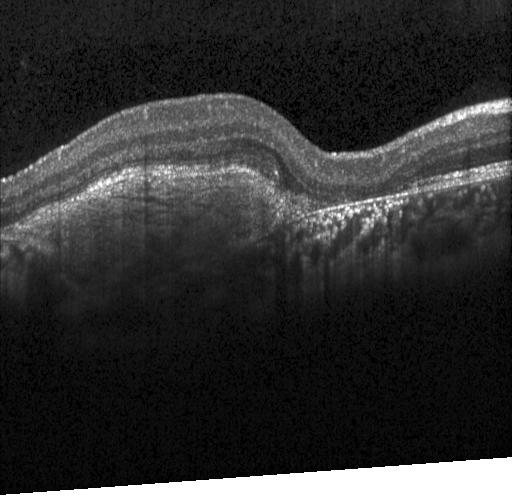
Optical coherence tomography B-scan.
Impression: choroidal neovascularization (CNV).